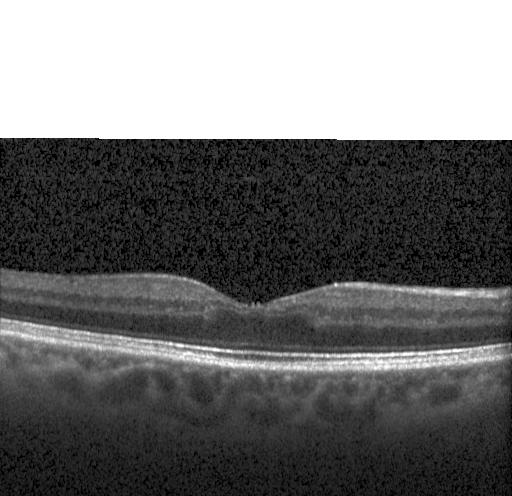
Retinal OCT B-scan.
The scan shows neither CNV, DME, nor drusen.